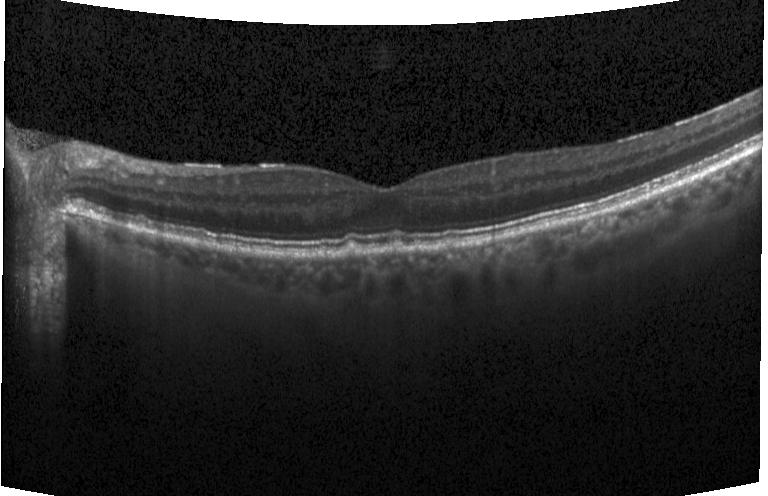

OCT B-scan showing drusen.